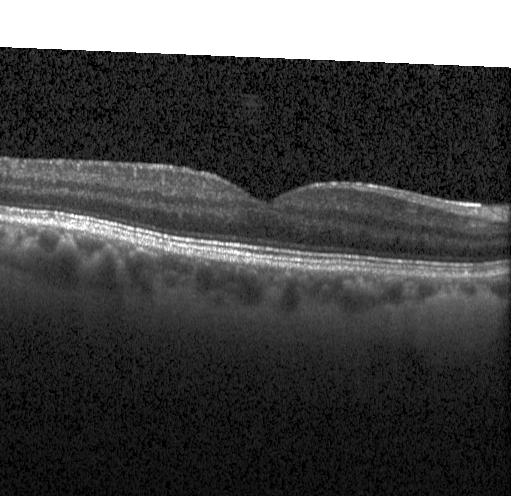

Spectral-domain optical coherence tomography. Through the macula. OCT B-scan. This B-scan demonstrates neither choroidal neovascularization, diabetic macular edema, nor drusen.